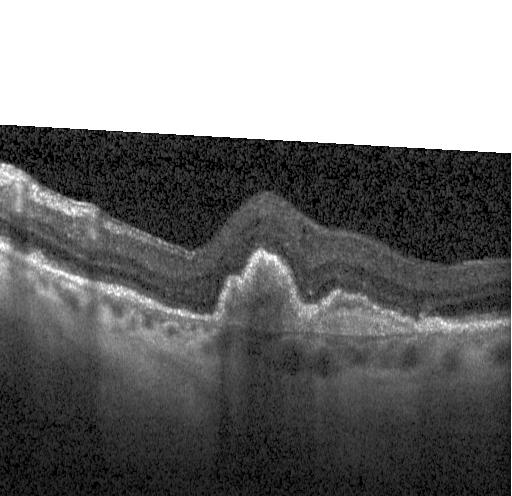

Macular OCT demonstrating a choroidal neovascular membrane.